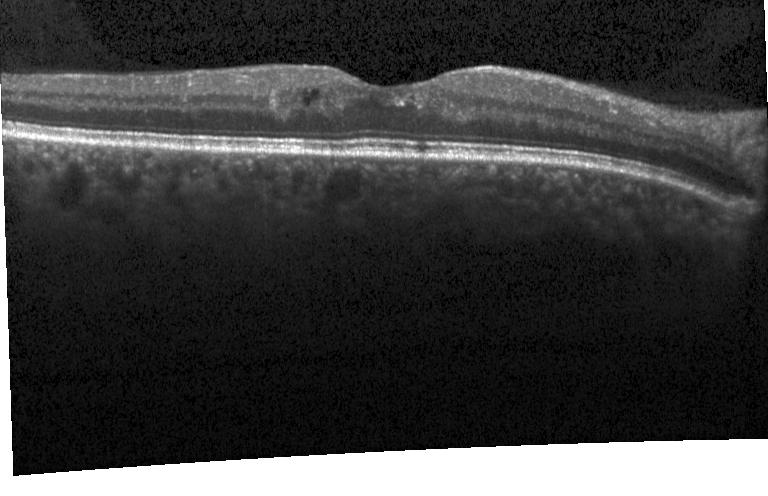 OCT scan showing diabetic macular edema.